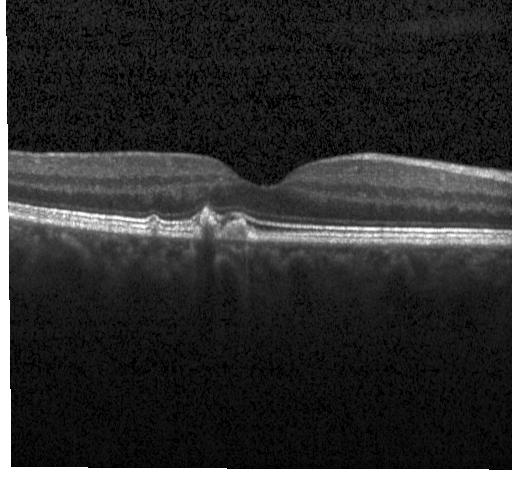
Optical coherence tomography scan. Assessment: sub-RPE drusenoid deposits.